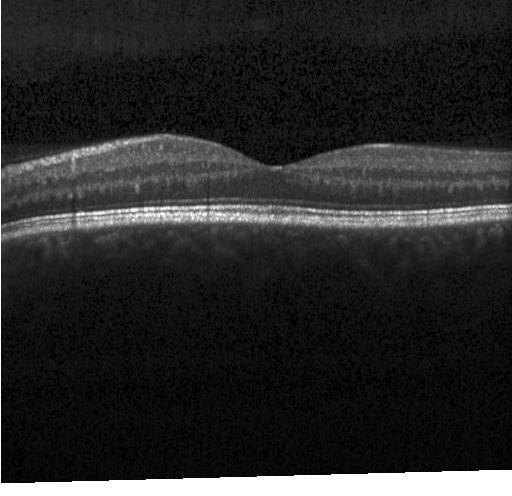 Macular OCT: no evidence of CNV, DME, or drusen.